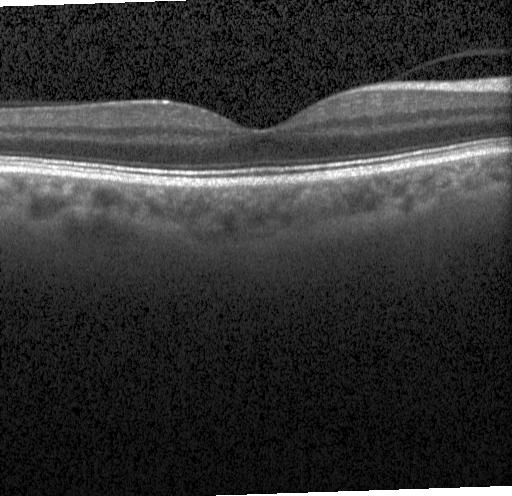

Dx: no evidence of CNV, DME, or drusen.